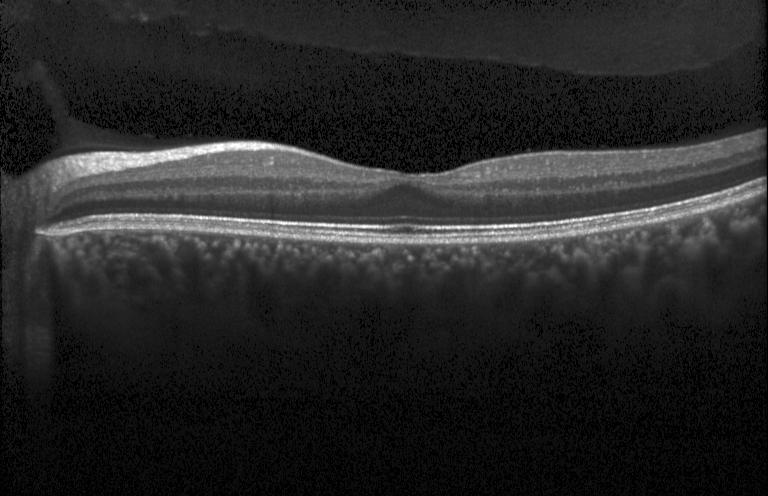 Macular OCT demonstrating neither choroidal neovascularization, diabetic macular edema, nor drusen.